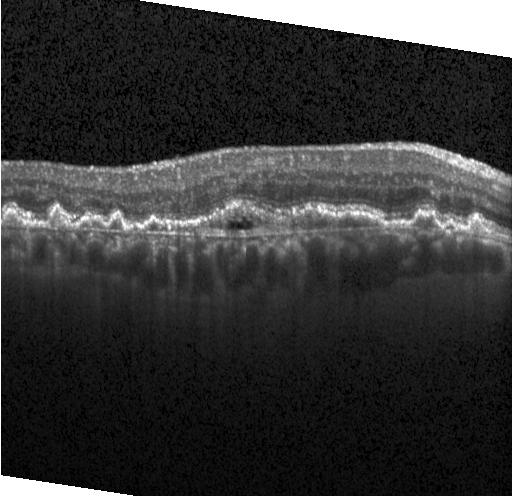

OCT line scan · Heidelberg Spectralis OCT system — Diagnosis: choroidal neovascularization.